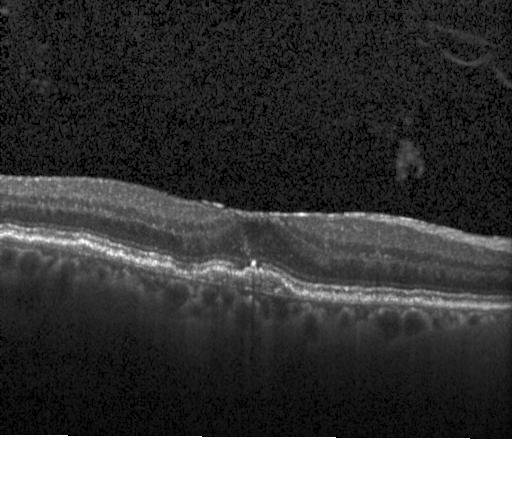

Retinal OCT B-scan. Macular OCT: choroidal neovascularization (CNV).